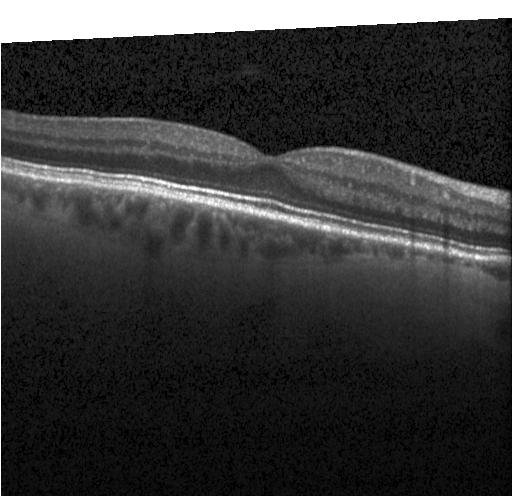

Acquired on a Heidelberg Spectralis · retinal OCT cross-section · spectral-domain OCT. Neither CNV, DME, nor drusen.